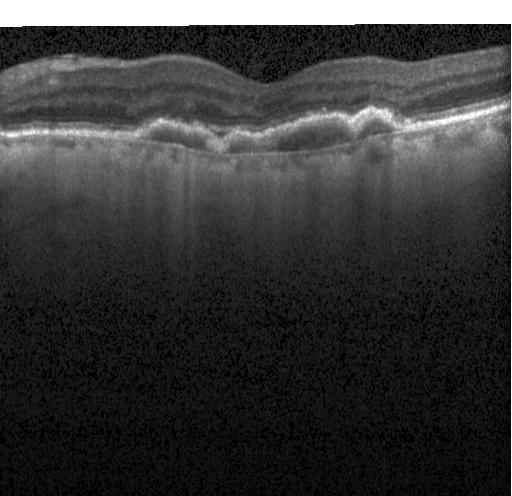
OCT B-scan showing choroidal neovascularization.